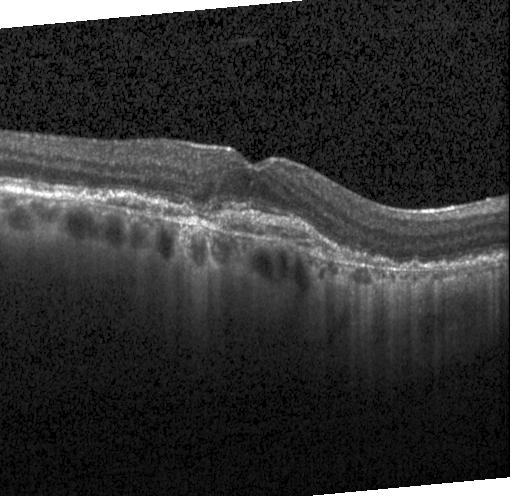
Impression: choroidal neovascularization (CNV).